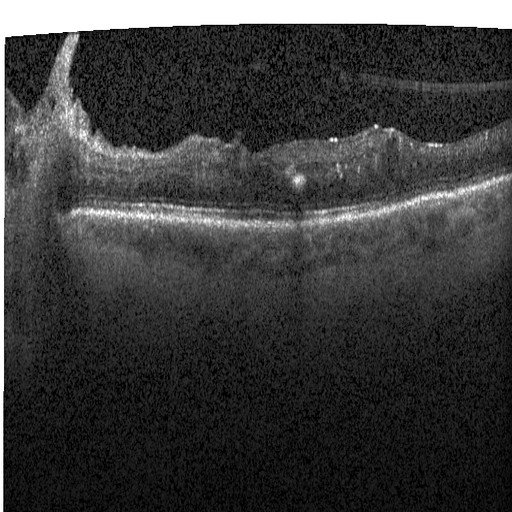 OCT line scan, acquired on a Heidelberg Spectralis — Finding: DME.